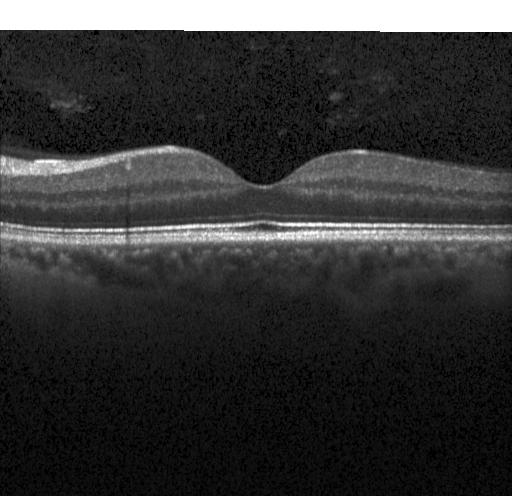

The scan shows no choroidal neovascularization, no diabetic macular edema, and no drusen.